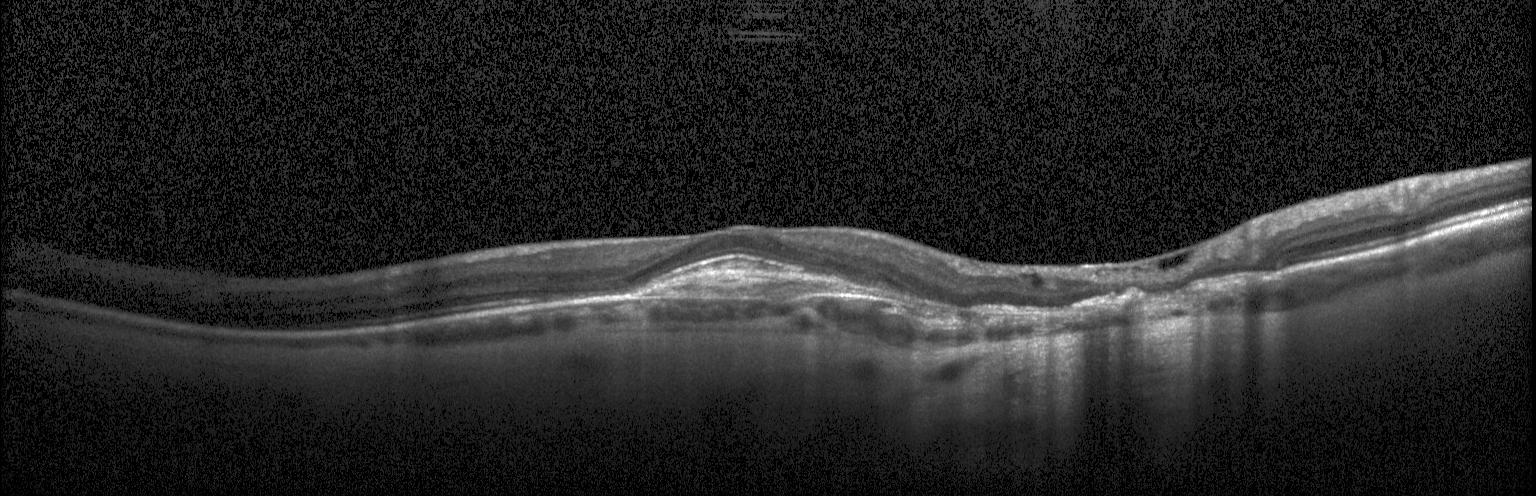
OCT line scan. Centered on the fovea — Macular OCT: a choroidal neovascular membrane.